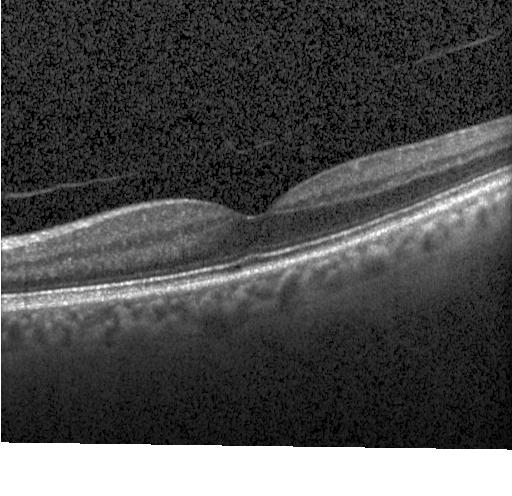 OCT B-scan; Heidelberg Spectralis OCT system; SD-OCT.
Impression: neither CNV, DME, nor drusen.